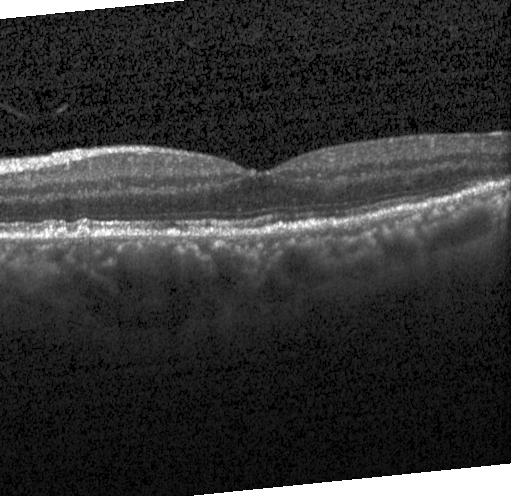 Through the macula · OCT B-scan · Heidelberg Spectralis OCT system. Diagnosis: multiple drusen.